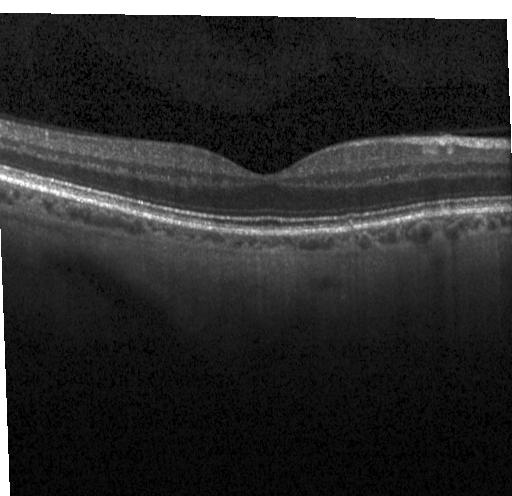
Horizontal scan through the fovea, OCT B-scan. Dx: neither choroidal neovascularization, diabetic macular edema, nor drusen.